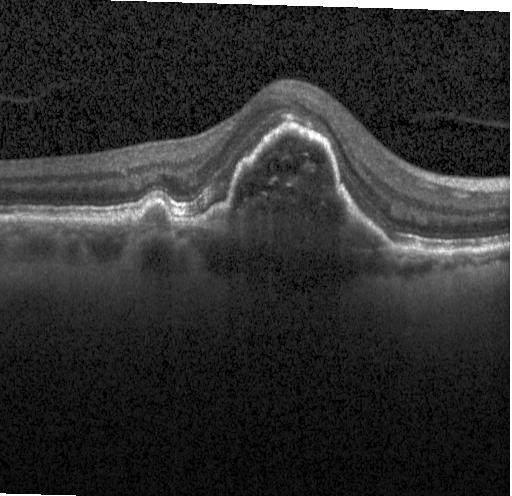 Dx: a choroidal neovascular membrane.